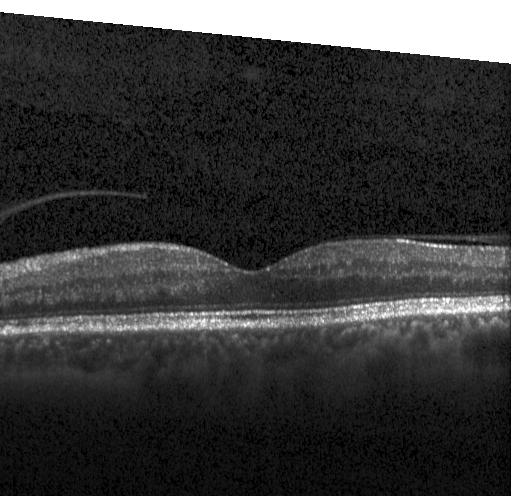

Retinal OCT cross-section.
OCT finding: neither CNV, DME, nor drusen.